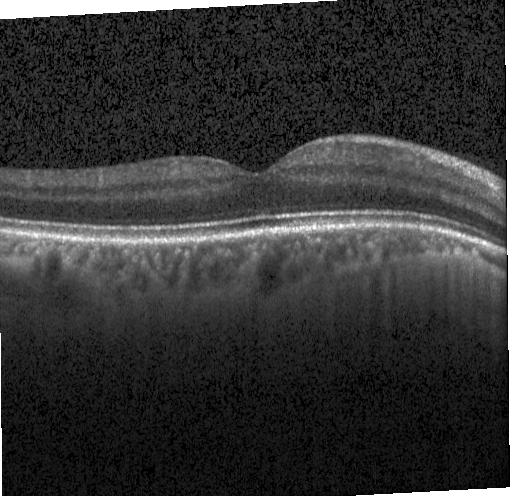
Finding: neither choroidal neovascularization, diabetic macular edema, nor drusen.